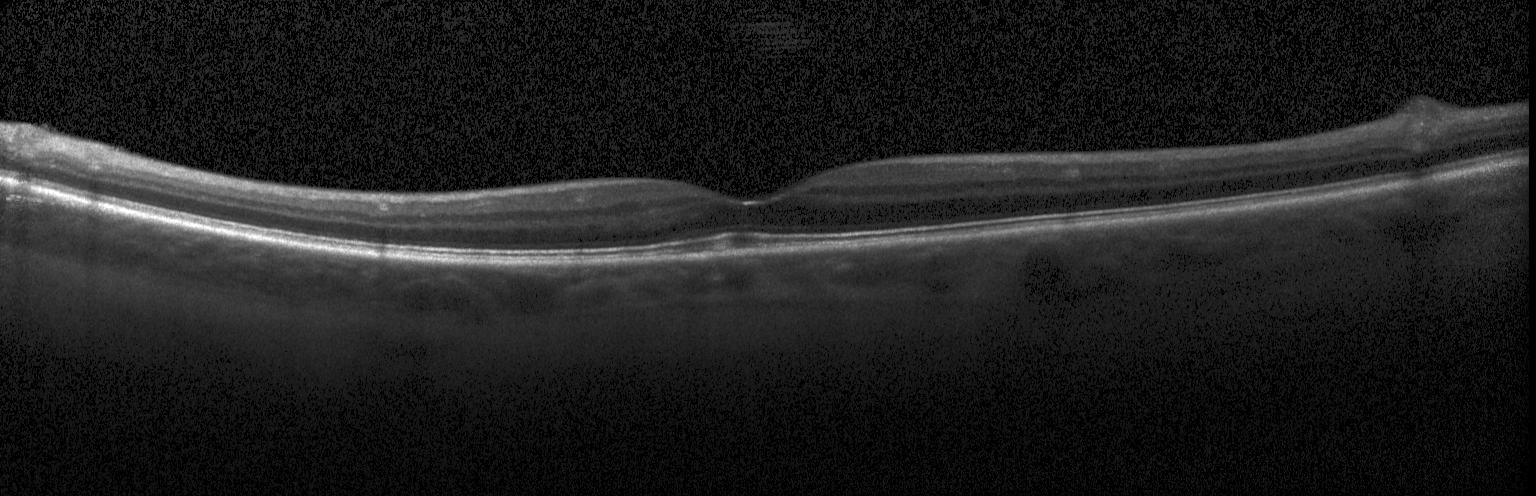

No choroidal neovascularization, no diabetic macular edema, and no drusen.